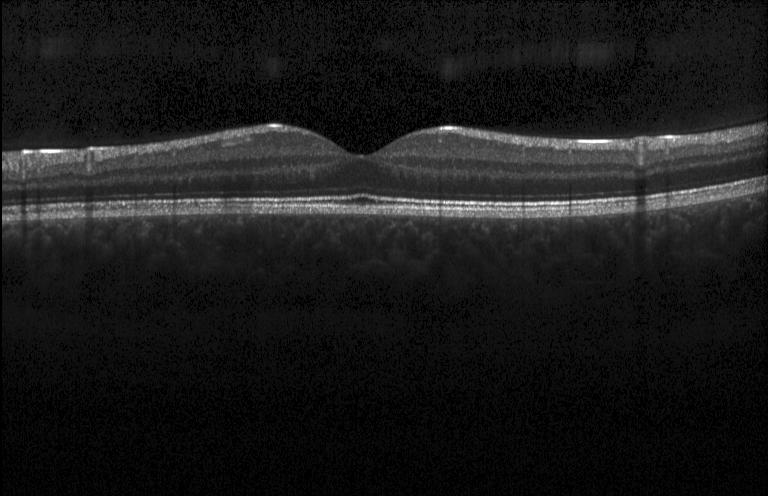

OCT B-scan showing no CNV, no DME, and no drusen.